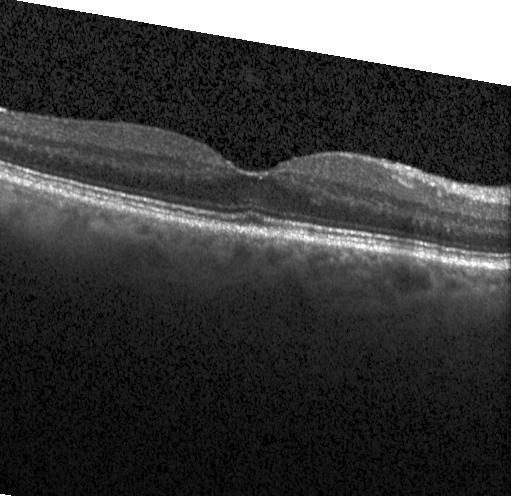 Optical coherence tomography B-scan · Heidelberg Spectralis OCT system · fovea-centered · spectral-domain OCT. This B-scan demonstrates no evidence of CNV, DME, or drusen.